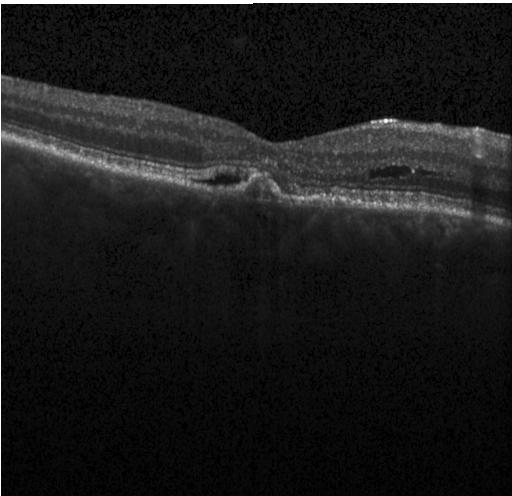

OCT B-scan.
Macular OCT: a choroidal neovascular membrane.